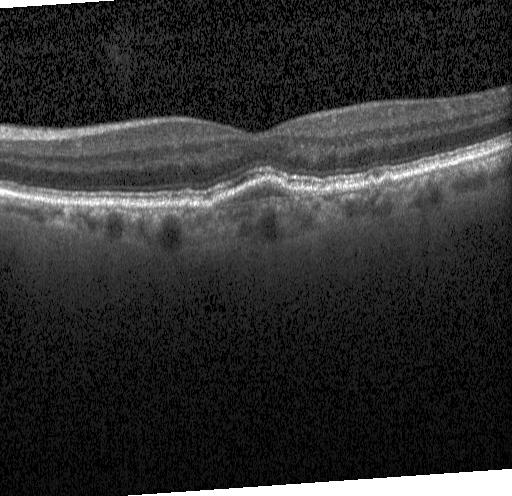 Dx: CNV.